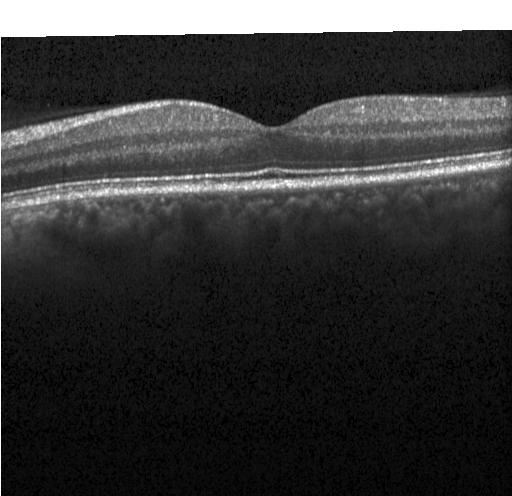
Retinal OCT cross-section showing no choroidal neovascularization, diabetic macular edema, or drusen.